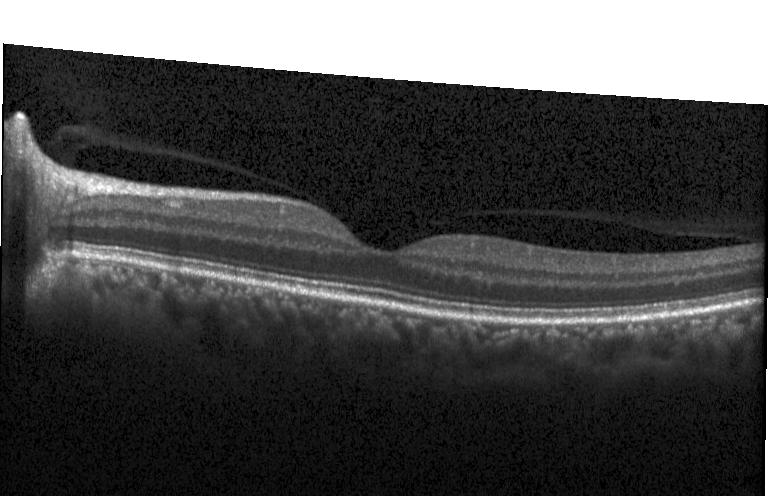 Finding: neither choroidal neovascularization, diabetic macular edema, nor drusen.